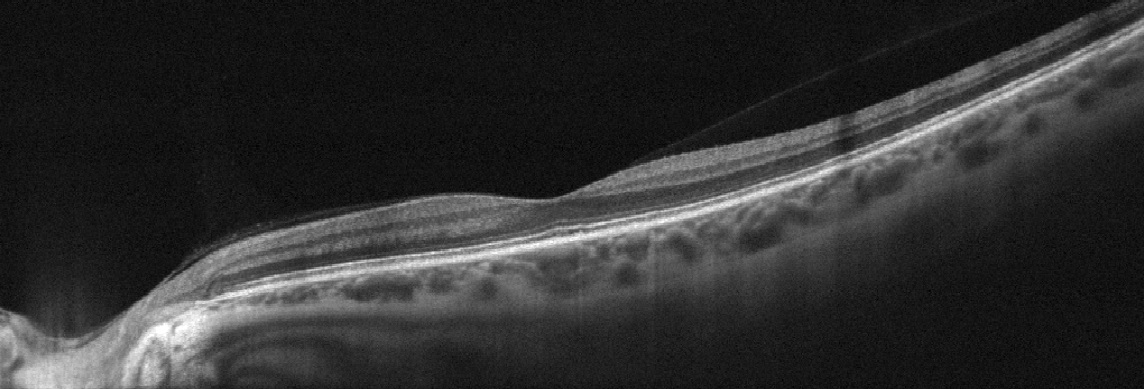 Diagnosis: no AMD, DME, ERM, RAO, RVO, or VID.